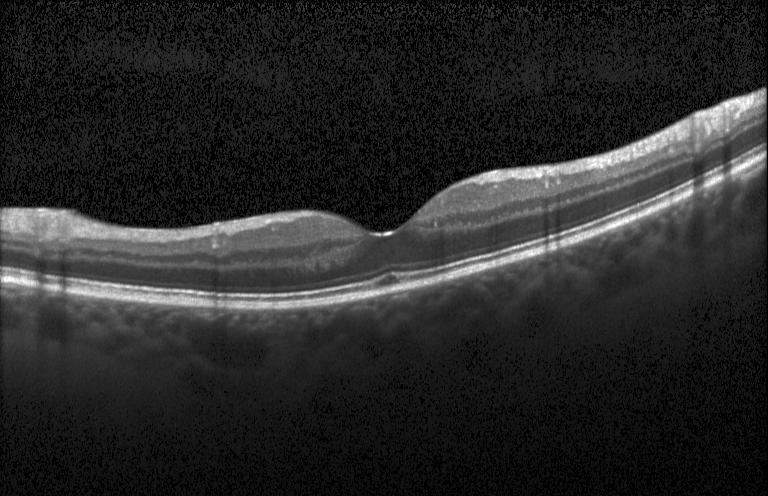 Spectral-domain OCT B-scan: no choroidal neovascularization, no diabetic macular edema, and no drusen.